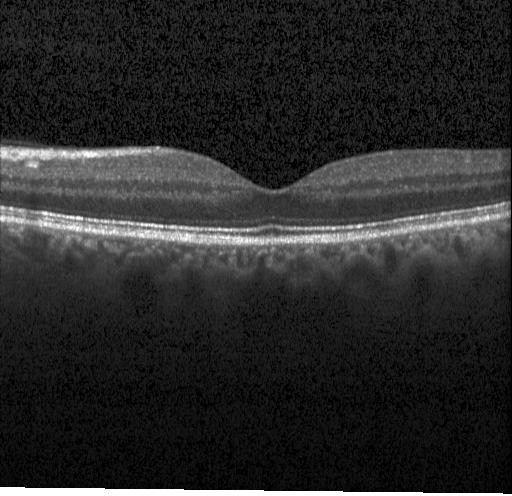

Centered on the fovea. OCT B-scan. SD-OCT. Acquired on a Heidelberg Spectralis — Neither CNV, DME, nor drusen.